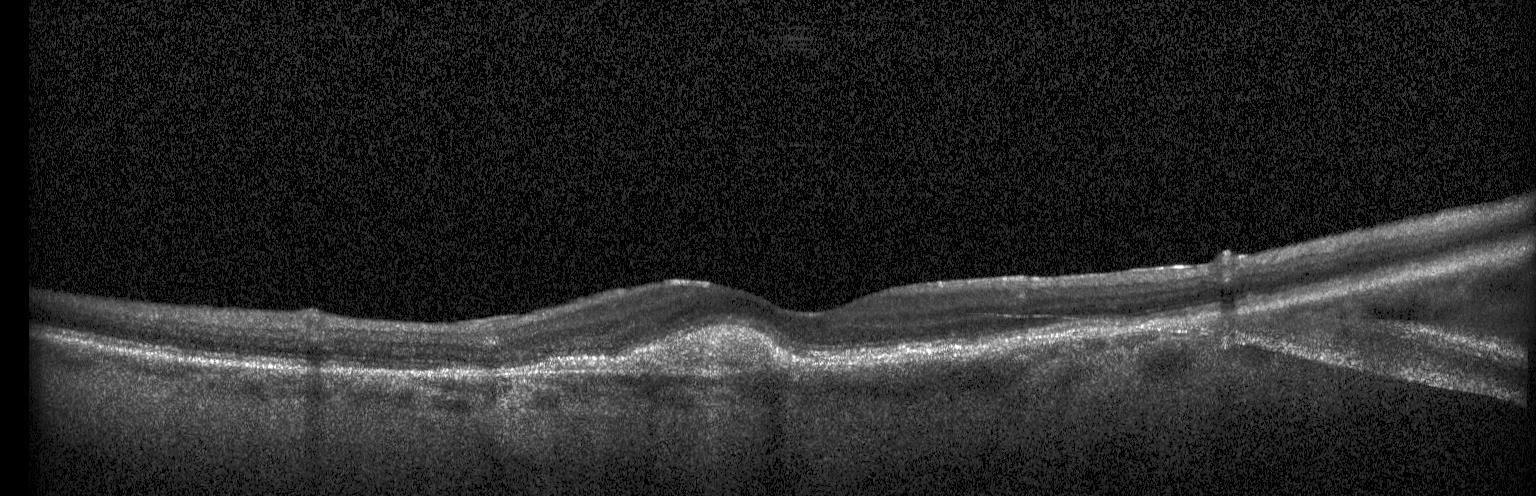

Macular OCT demonstrating a choroidal neovascular membrane.